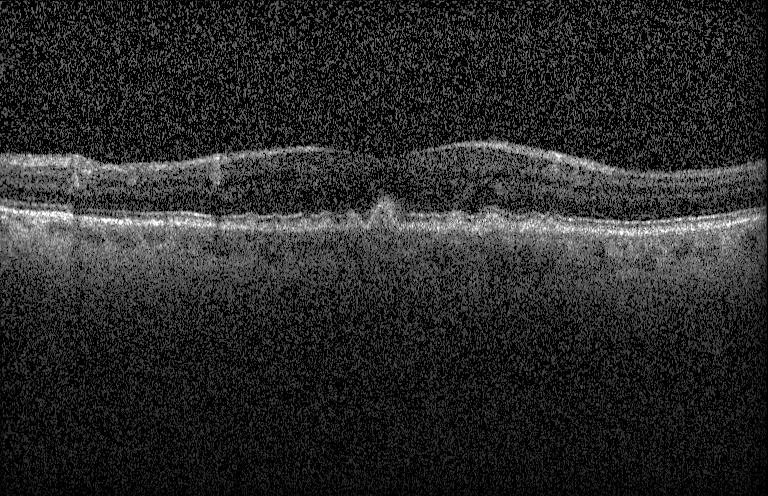 The scan shows multiple drusen.